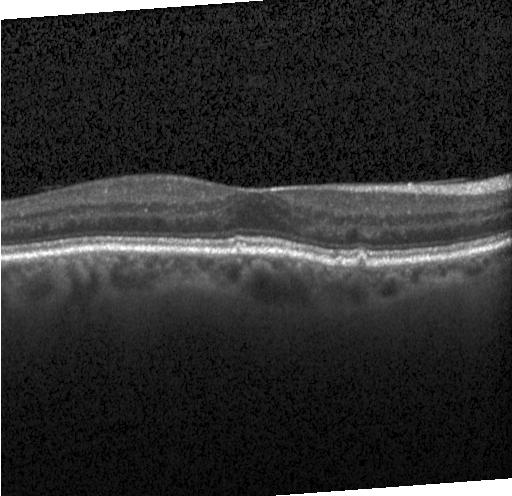 OCT B-scan · fovea-centered · SD-OCT · Heidelberg Spectralis — Impression: drusen.